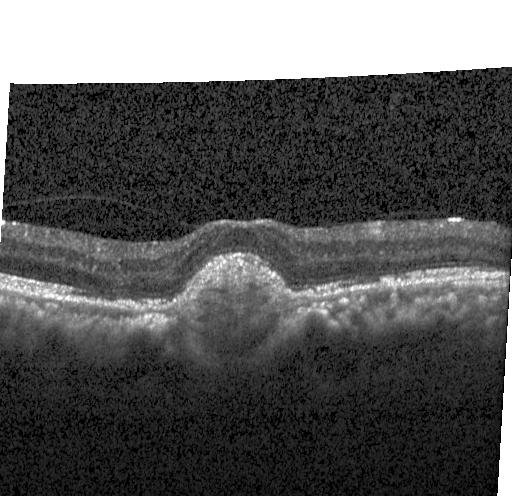 Acquired on a Heidelberg Spectralis, spectral-domain OCT, retinal OCT cross-section
A choroidal neovascular membrane.